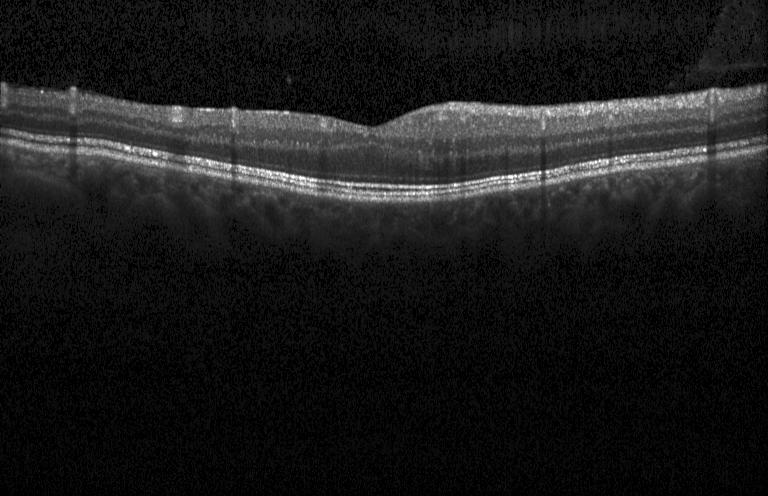

SD-OCT; optical coherence tomography B-scan; Heidelberg Spectralis; centered on the fovea — Diagnosis: neither choroidal neovascularization, diabetic macular edema, nor drusen.